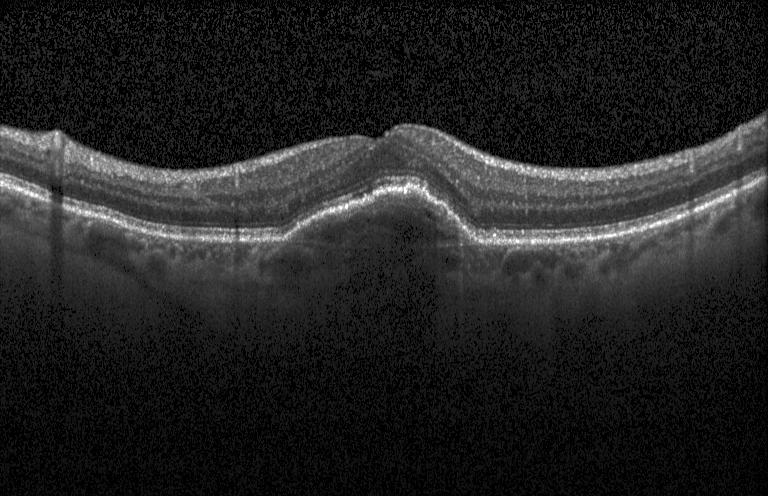
This B-scan demonstrates choroidal neovascularization (CNV).